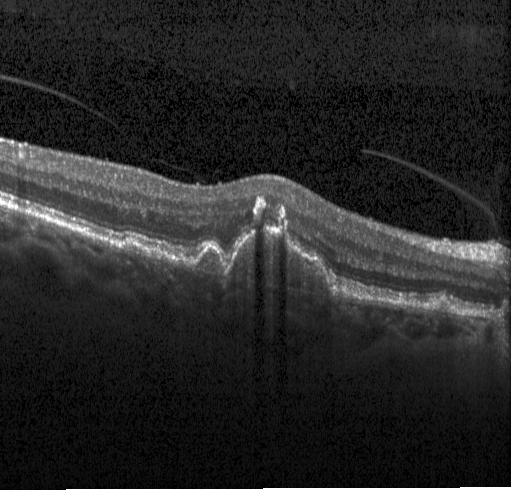
OCT B-scan.
Choroidal neovascularization (CNV).